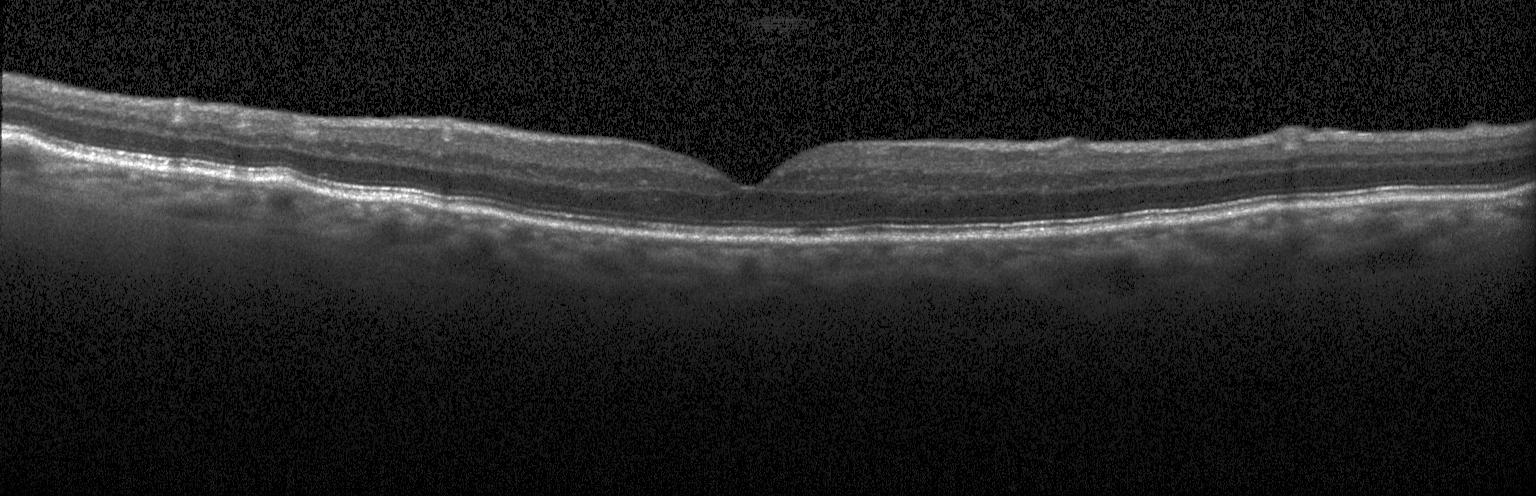 Finding: no choroidal neovascularization, no diabetic macular edema, and no drusen.